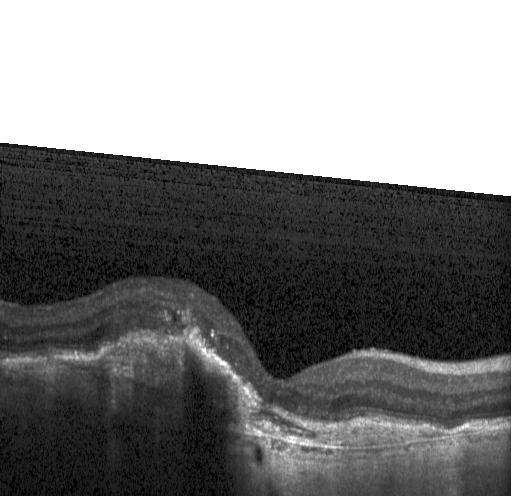

OCT finding: a choroidal neovascular membrane.